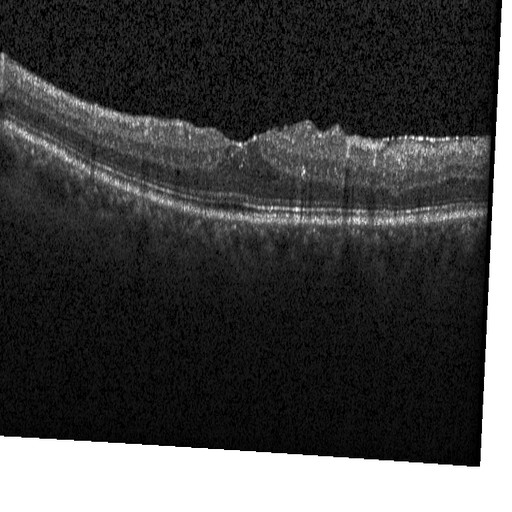

Spectral-domain optical coherence tomography · optical coherence tomography scan — Finding: DME.